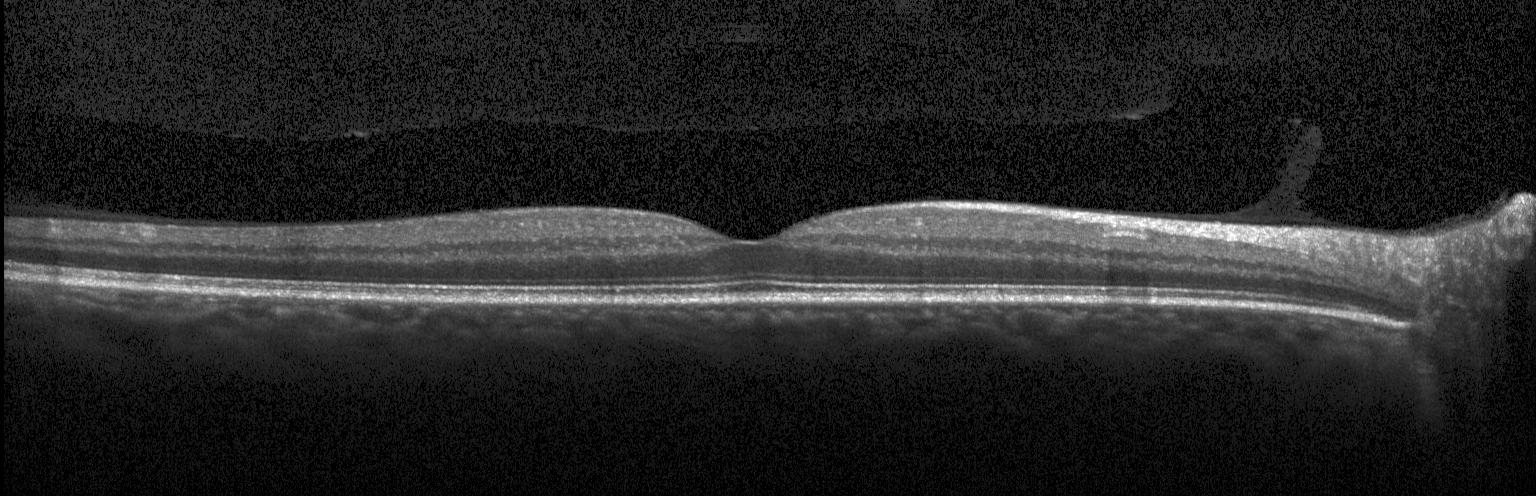

OCT finding: no evidence of CNV, DME, or drusen.